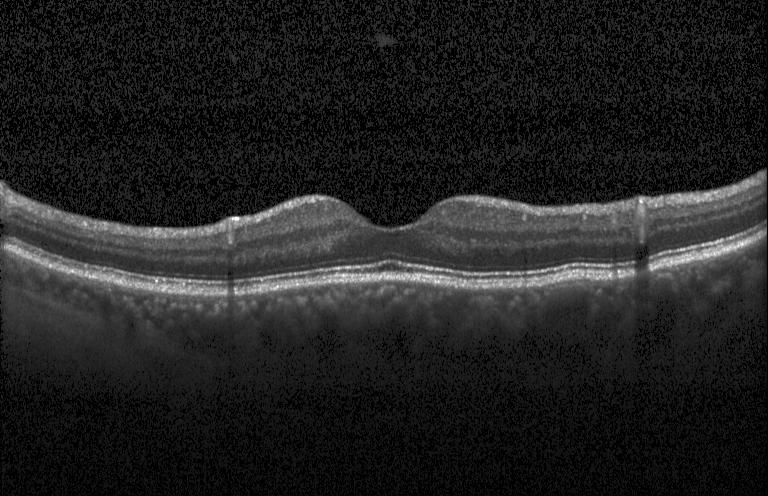

OCT line scan.
Finding: no CNV, DME, or drusen.